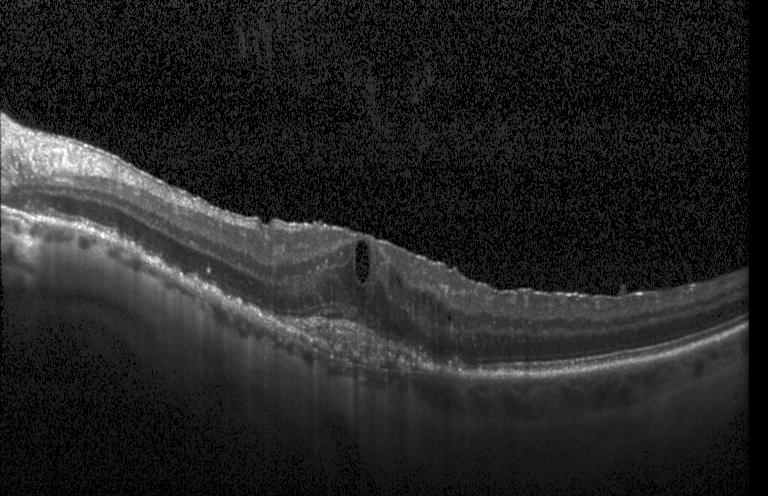
Instrument: Heidelberg Spectralis; retinal OCT B-scan; spectral-domain OCT; horizontal scan through the fovea
Dx: CNV.